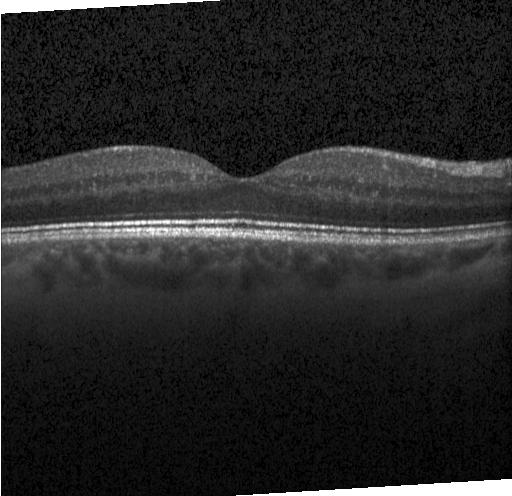 OCT finding: no choroidal neovascularization, no diabetic macular edema, and no drusen.